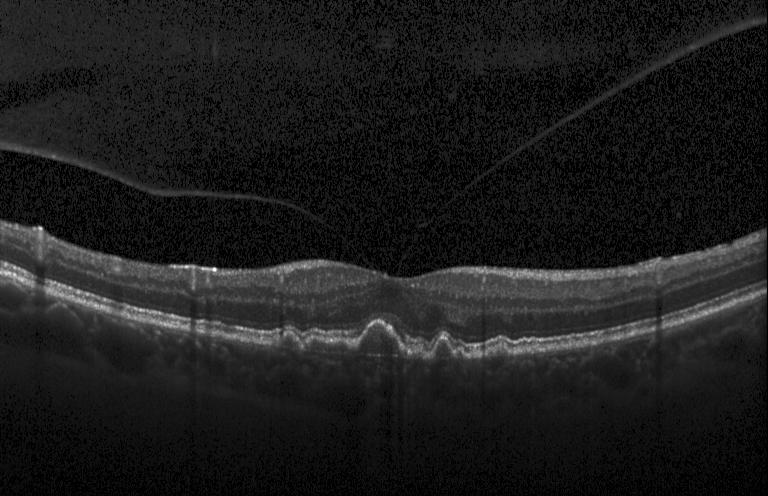
Macular OCT demonstrating multiple drusen.